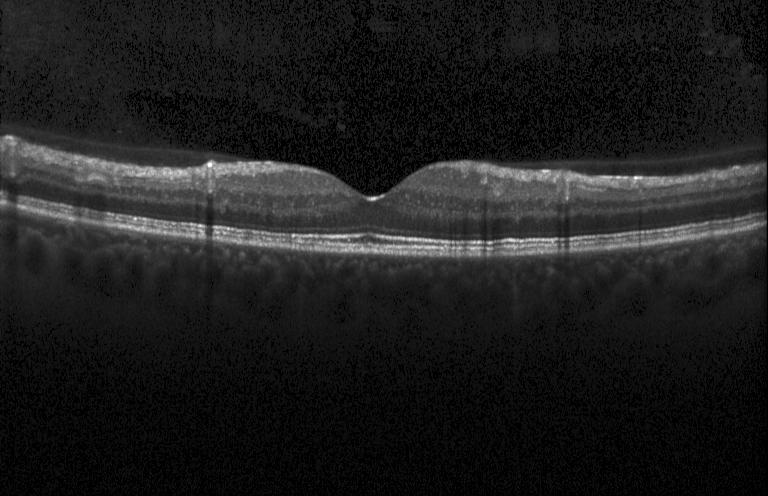

OCT finding: no CNV, DME, or drusen.